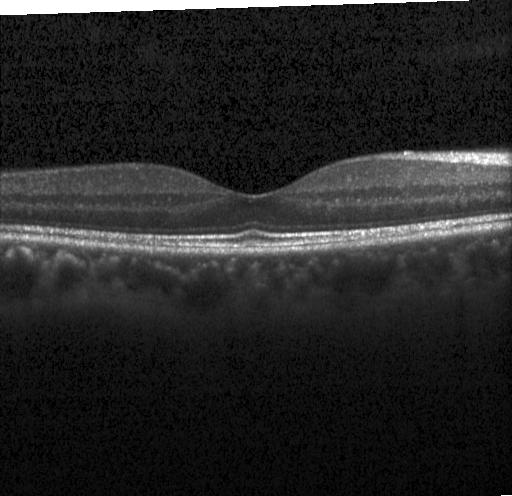 Macular OCT: no choroidal neovascularization, no diabetic macular edema, and no drusen.